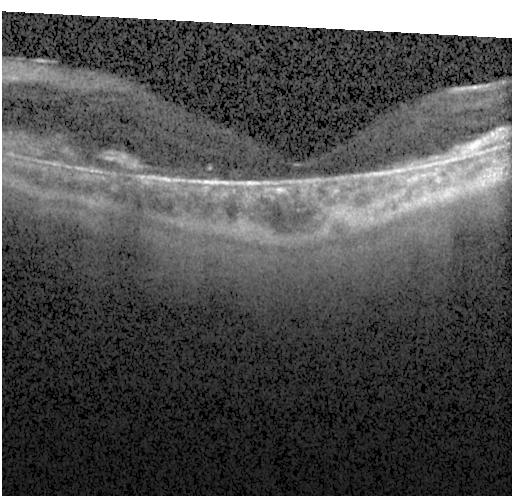 Finding: CNV.